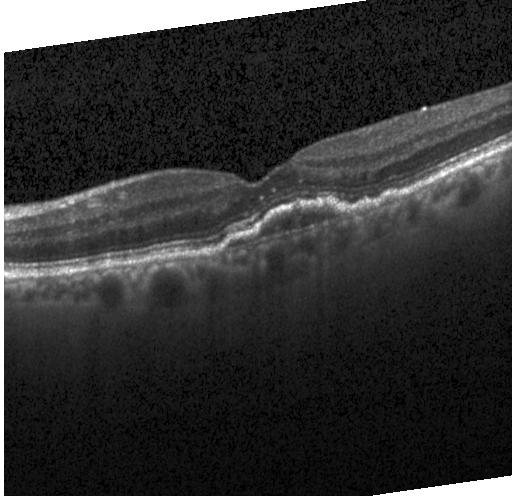 Optical coherence tomography B-scan.
This B-scan demonstrates CNV.